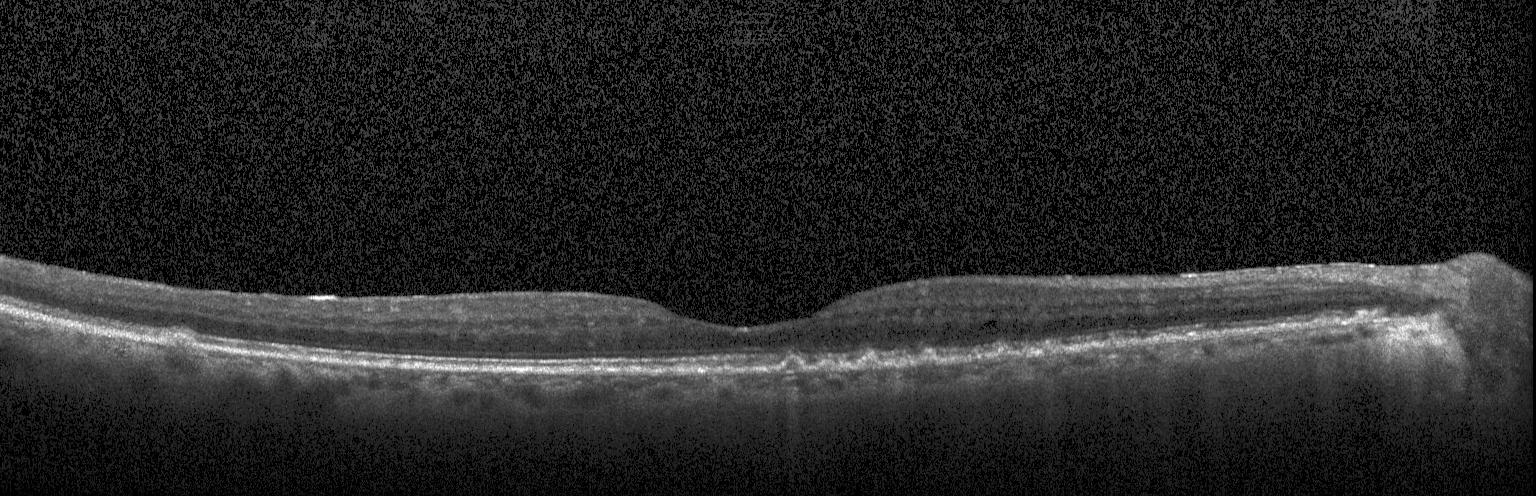 Centered on the fovea. Retinal OCT cross-section — Finding: sub-RPE drusenoid deposits.